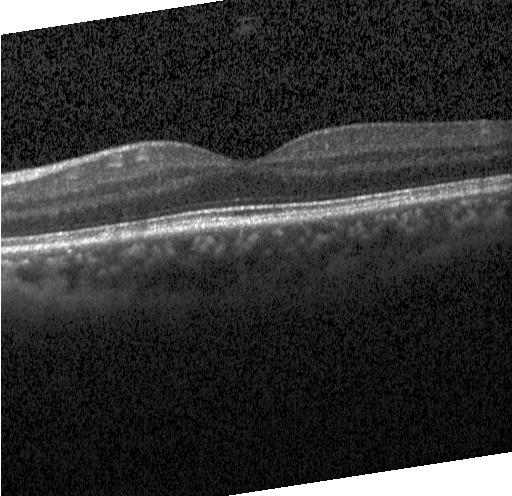
Dx: neither choroidal neovascularization, diabetic macular edema, nor drusen.